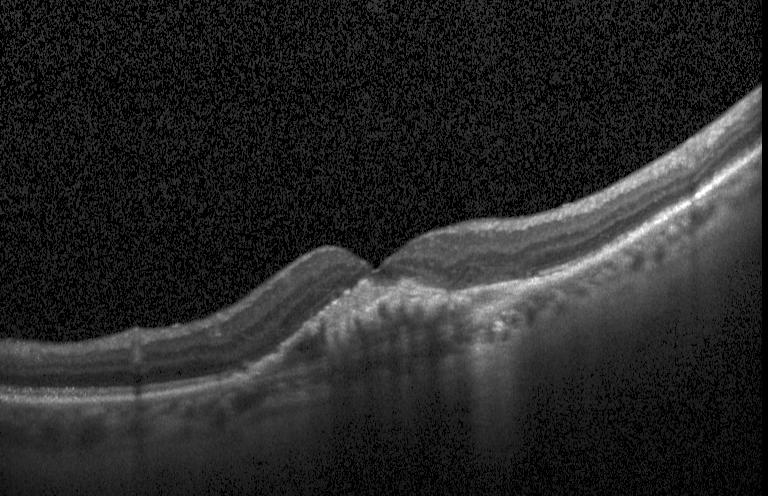 Macular OCT: a choroidal neovascular membrane.